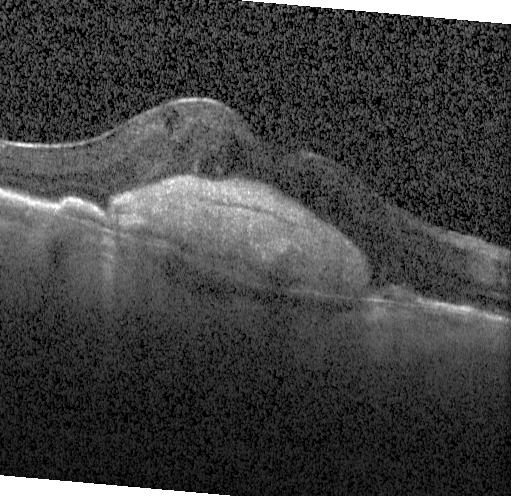

Impression: choroidal neovascularization.